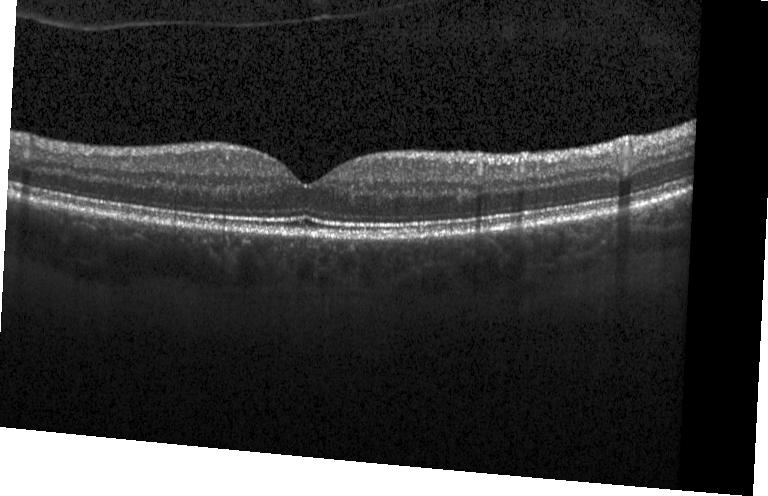

Retinal OCT cross-section
Macular OCT: no evidence of choroidal neovascularization, diabetic macular edema, or drusen.